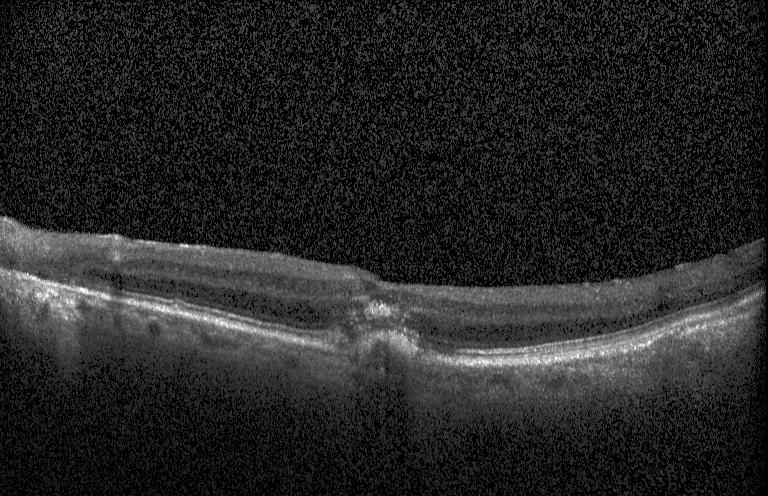
Finding: choroidal neovascularization (CNV).